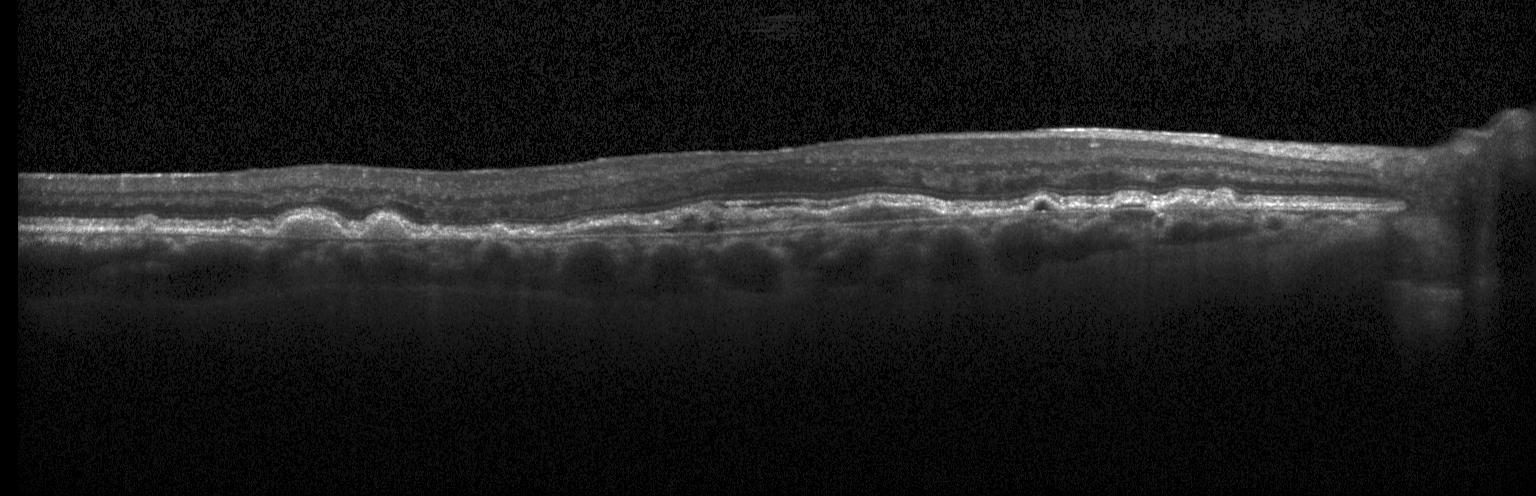
Retinal OCT cross-section showing choroidal neovascularization.